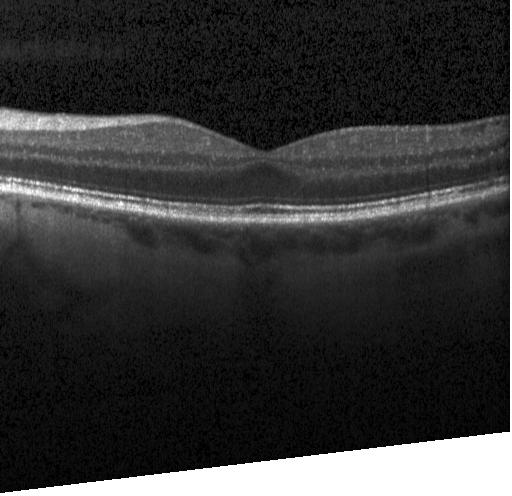

OCT line scan; Heidelberg Spectralis. Dx: no evidence of choroidal neovascularization, diabetic macular edema, or drusen.